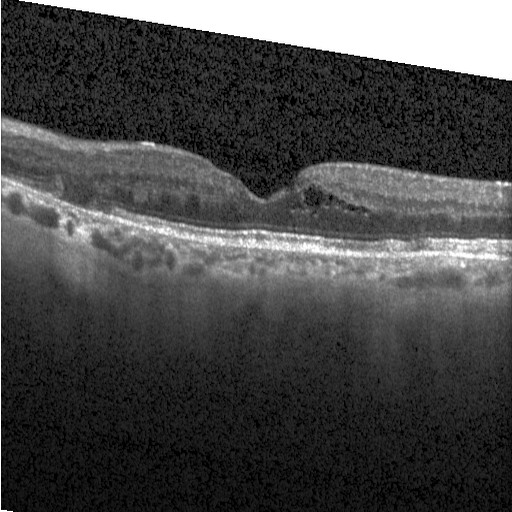 Spectral-domain OCT; retinal OCT B-scan; horizontal scan through the fovea; acquired on a Heidelberg Spectralis.
This B-scan demonstrates diabetic macular edema (DME).